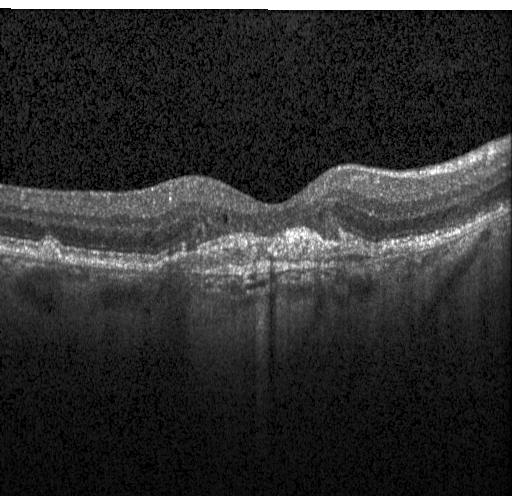

Spectral-domain OCT; optical coherence tomography scan; Heidelberg Spectralis; horizontal scan through the fovea. Assessment: a choroidal neovascular membrane.